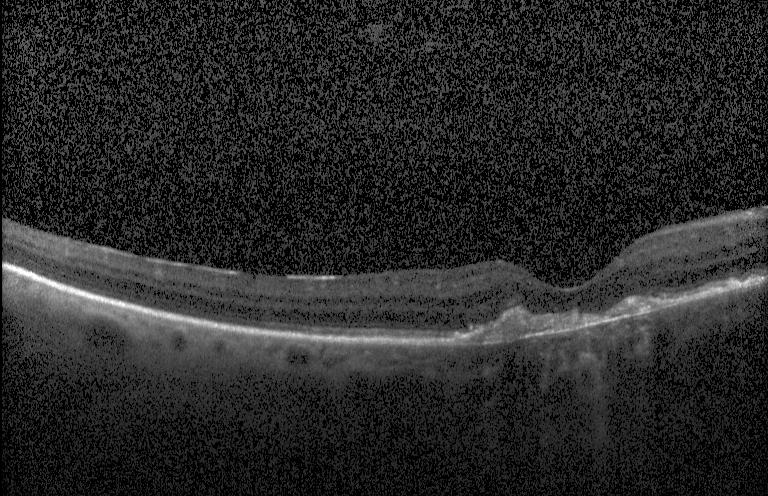 SD-OCT · OCT line scan — The scan shows a choroidal neovascular membrane.